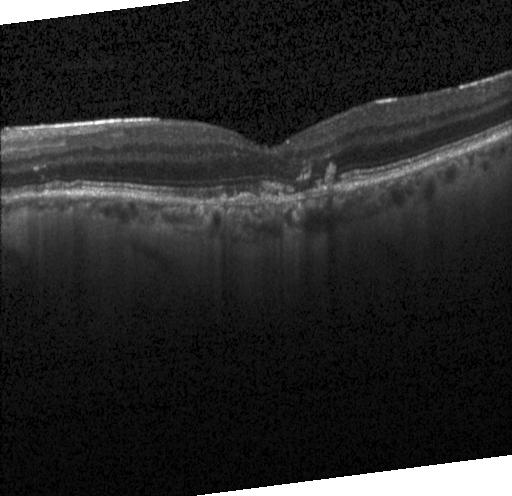 The scan shows CNV.